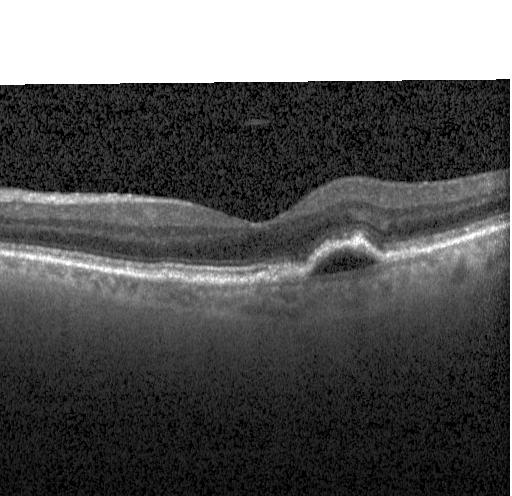
Macular OCT: CNV.